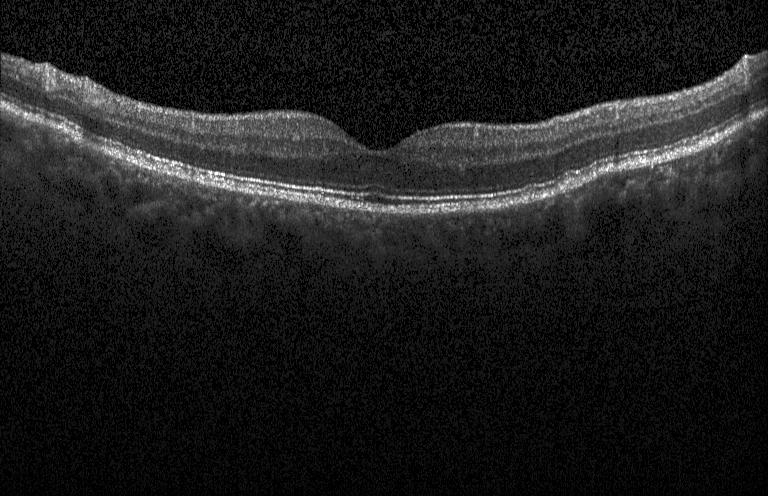

OCT B-scan showing neither CNV, DME, nor drusen.